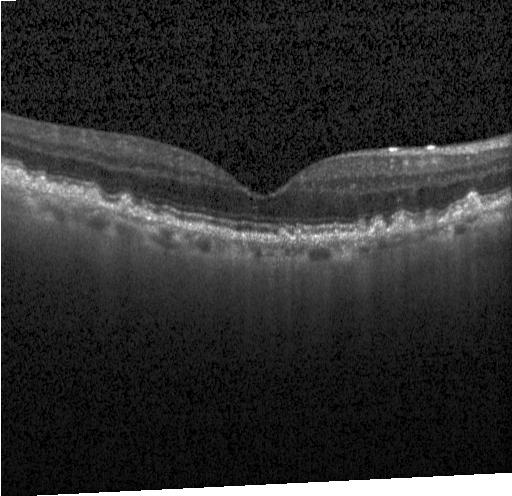

Heidelberg Spectralis OCT system, centered on the fovea, optical coherence tomography scan — Assessment: drusen.